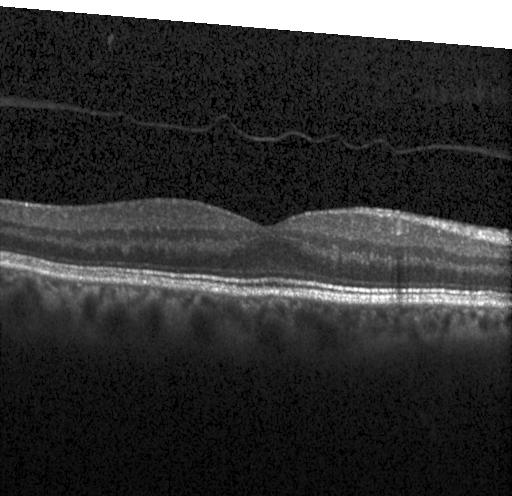
Optical coherence tomography B-scan — Impression: neither choroidal neovascularization, diabetic macular edema, nor drusen.